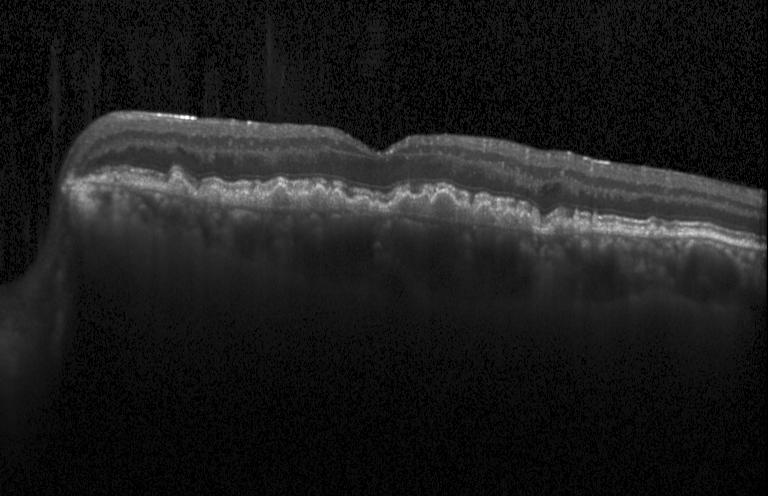

Centered on the fovea. Spectral-domain OCT. OCT line scan — This B-scan demonstrates a choroidal neovascular membrane.